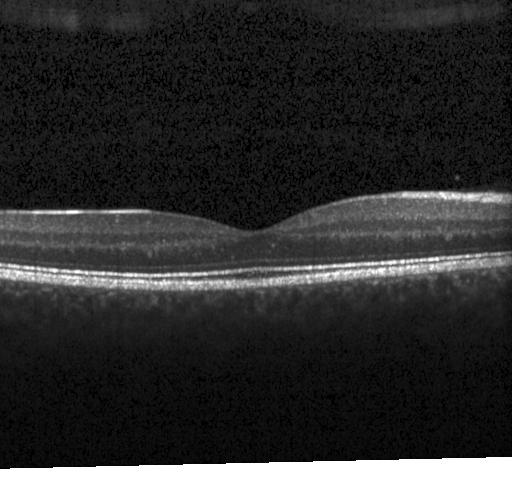 Assessment: no evidence of choroidal neovascularization, diabetic macular edema, or drusen.